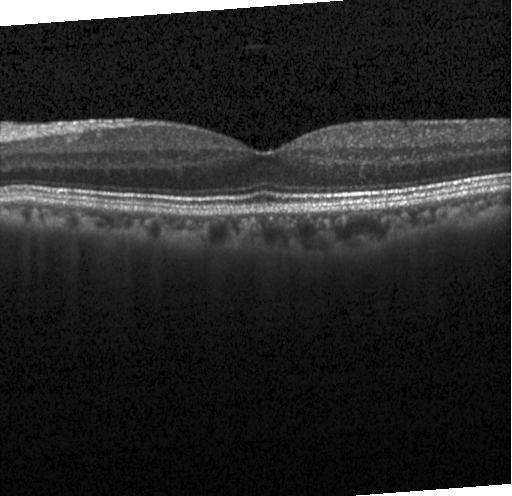
Optical coherence tomography scan. No choroidal neovascularization, no diabetic macular edema, and no drusen.